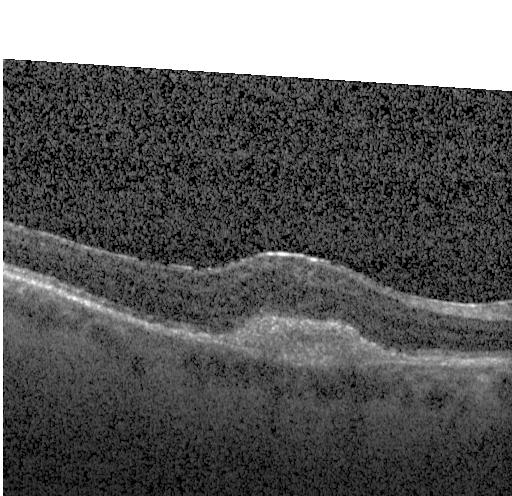 A choroidal neovascular membrane.